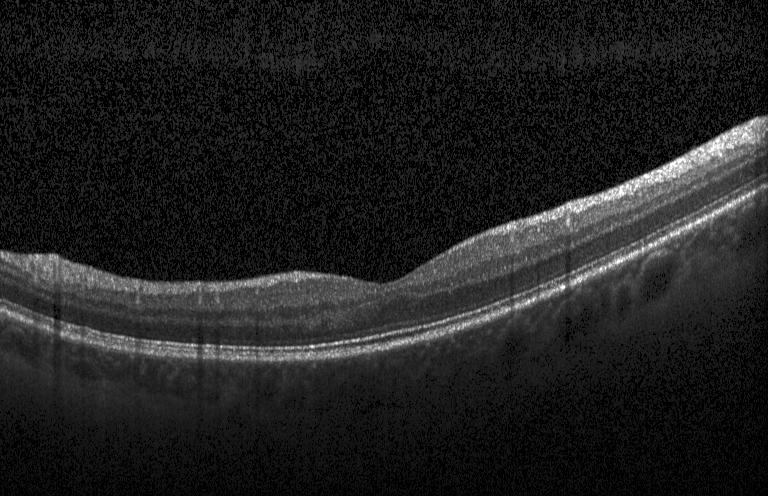

Retinal OCT B-scan. Diagnosis: no evidence of choroidal neovascularization, diabetic macular edema, or drusen.